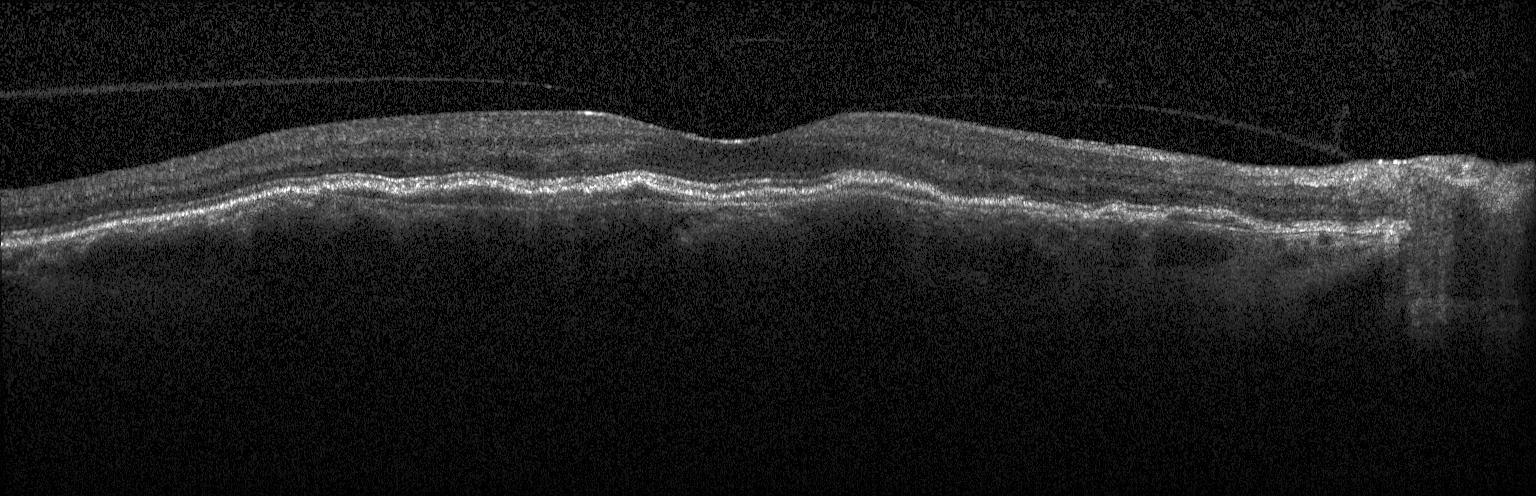
OCT B-scan. This B-scan demonstrates a choroidal neovascular membrane.